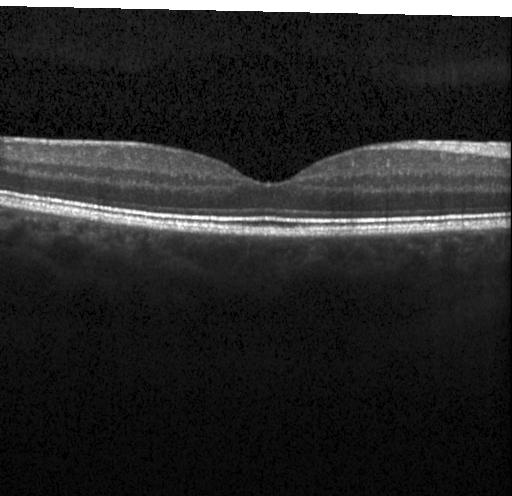 Finding: no CNV, no DME, and no drusen.